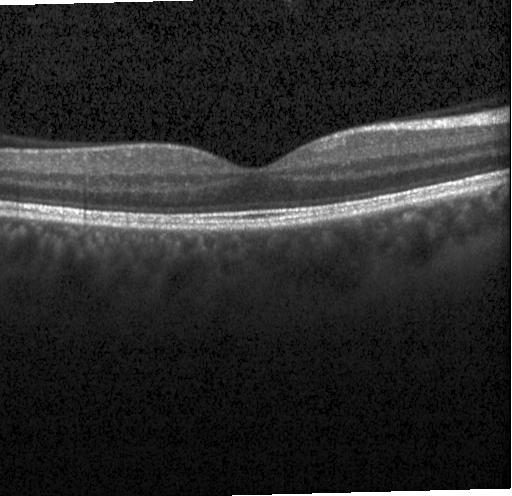
Fovea-centered; Heidelberg Spectralis OCT system; retinal OCT B-scan
Macular OCT: neither choroidal neovascularization, diabetic macular edema, nor drusen.